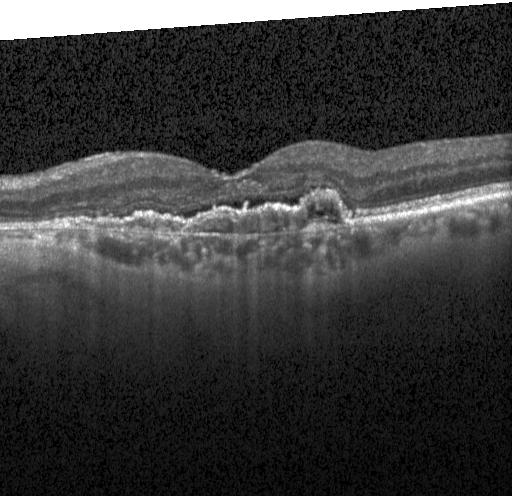 Optical coherence tomography B-scan — Diagnosis: a choroidal neovascular membrane.